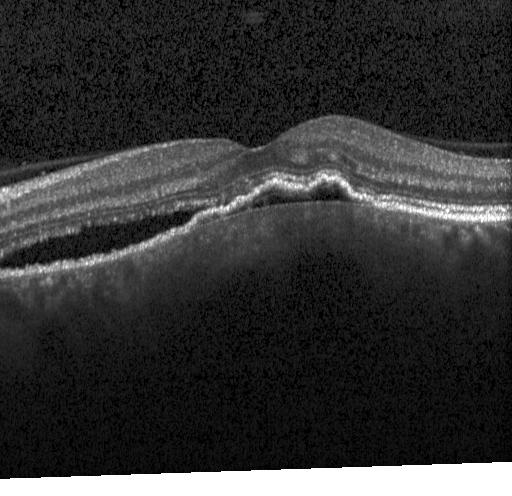

Finding: CNV.